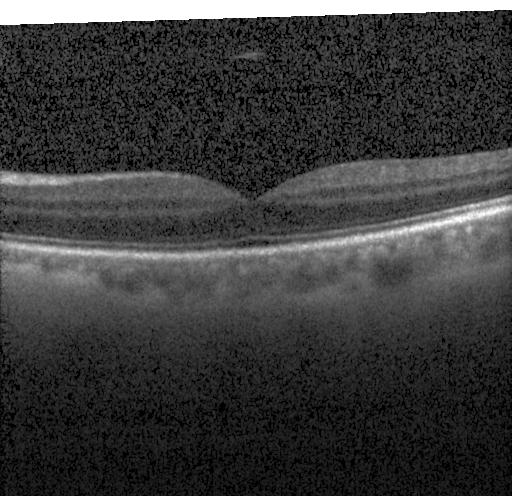 This B-scan demonstrates no choroidal neovascularization, no diabetic macular edema, and no drusen.